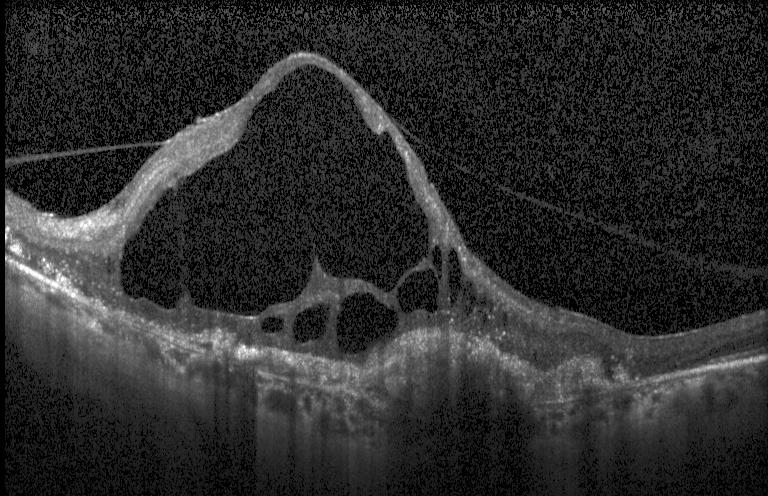 Assessment: a choroidal neovascular membrane.